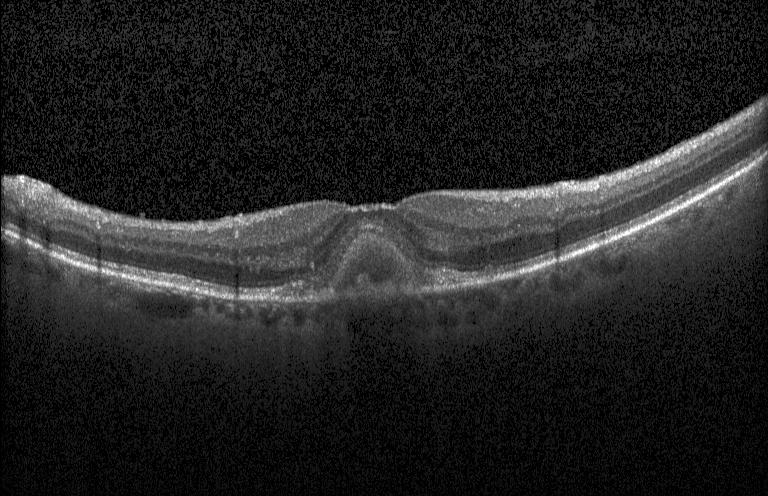 Retinal OCT B-scan
CNV.